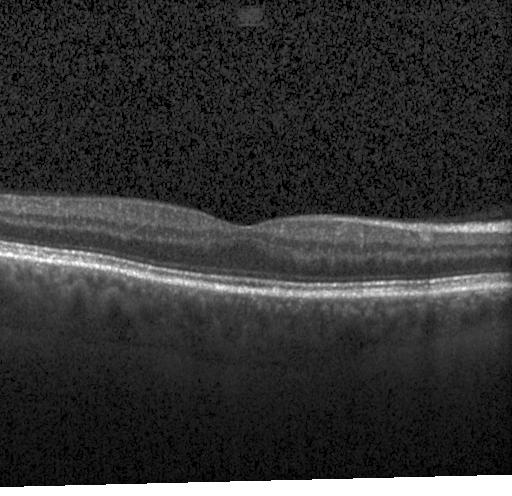 This B-scan demonstrates no choroidal neovascularization, diabetic macular edema, or drusen.